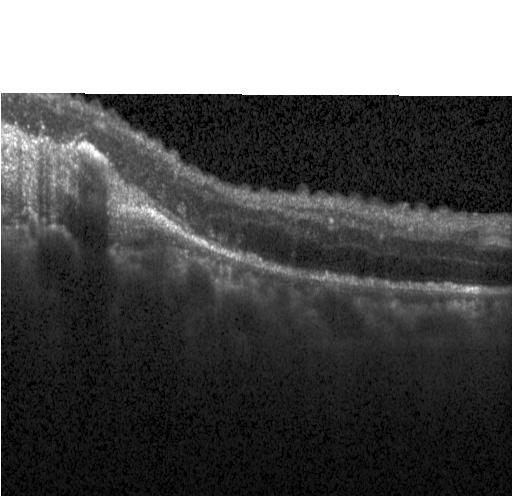 Retinal OCT cross-section. Through the macula. Spectral-domain OCT. Heidelberg Spectralis. A choroidal neovascular membrane.